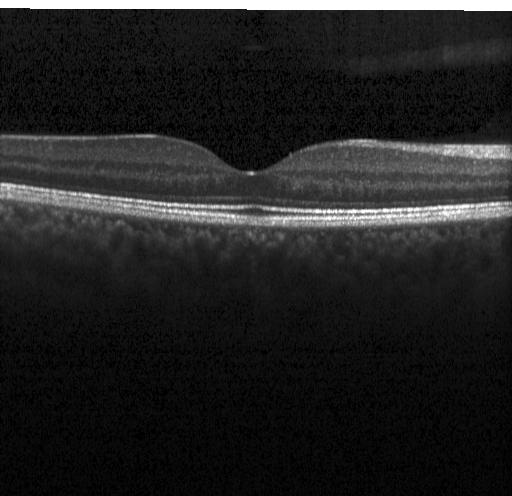 Retinal OCT B-scan
Finding: neither choroidal neovascularization, diabetic macular edema, nor drusen.